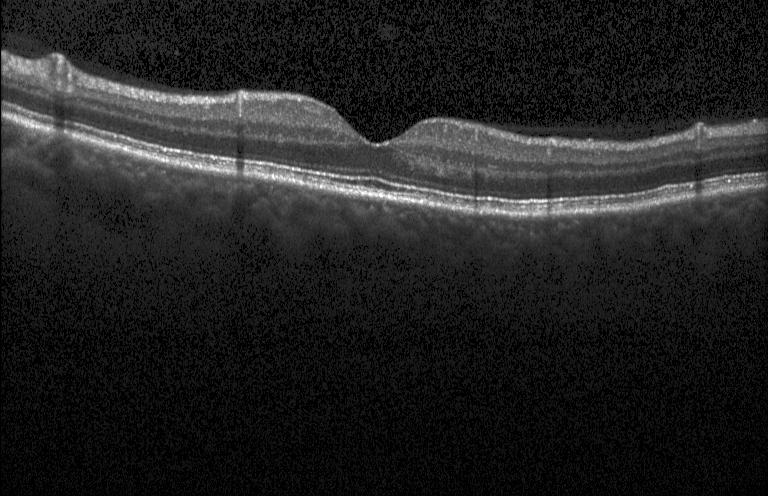
No evidence of choroidal neovascularization, diabetic macular edema, or drusen.